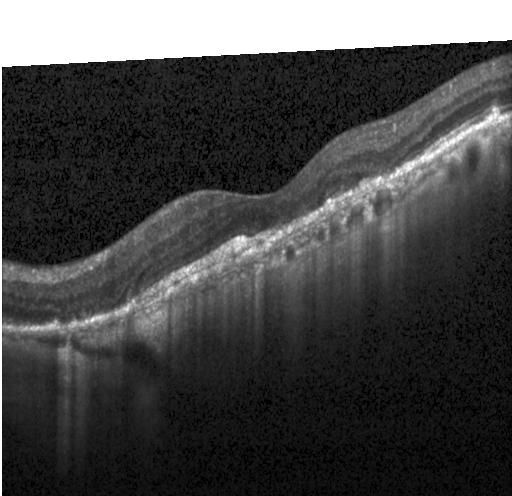
Retinal OCT B-scan; fovea-centered. The scan shows CNV.